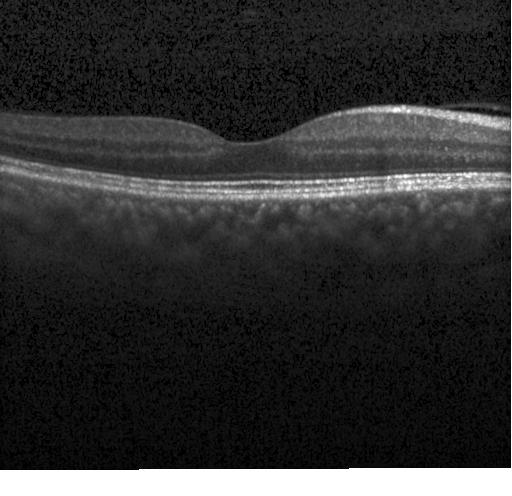

Optical coherence tomography scan — Diagnosis: no evidence of choroidal neovascularization, diabetic macular edema, or drusen.